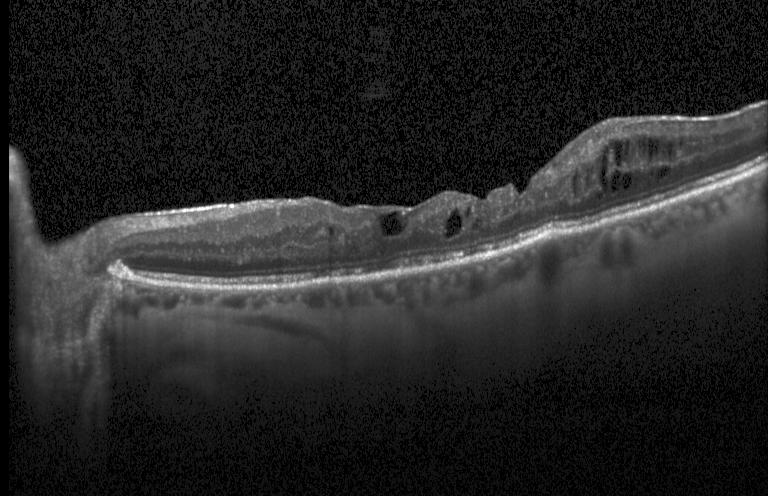
Retinal OCT cross-section, instrument: Heidelberg Spectralis, fovea-centered.
Diagnosis: diabetic macular edema.